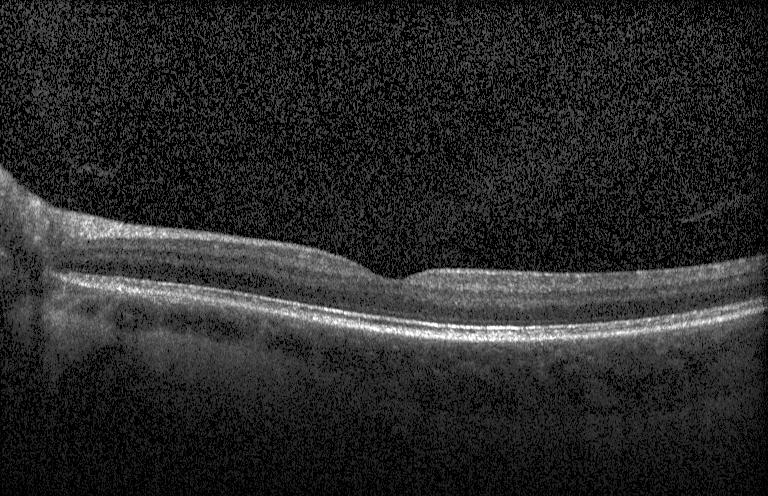

OCT line scan, SD-OCT — Finding: no choroidal neovascularization, diabetic macular edema, or drusen.